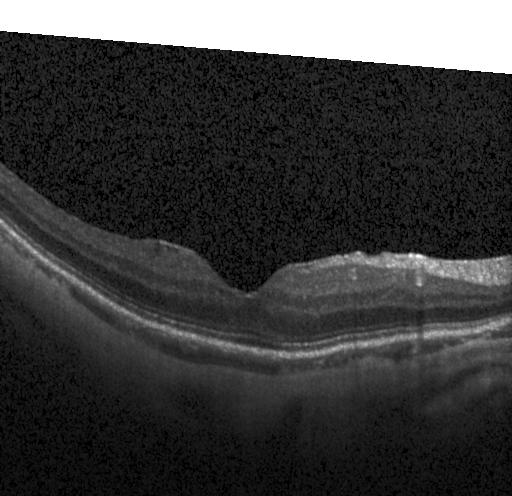

Macular OCT: no CNV, DME, or drusen.